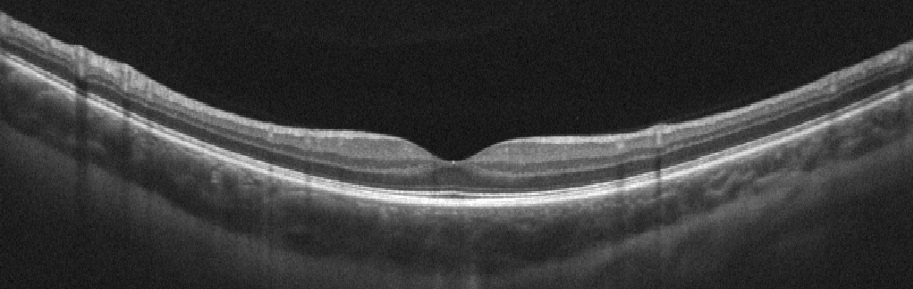

Spectral-domain OCT B-scan: absence of AMD, DME, ERM, RAO, RVO, and vitreomacular interface disease.